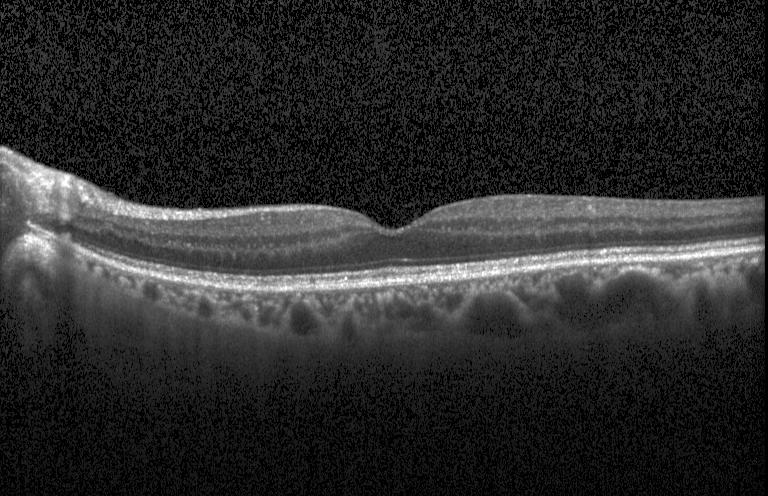

OCT line scan. Heidelberg Spectralis — Finding: neither CNV, DME, nor drusen.